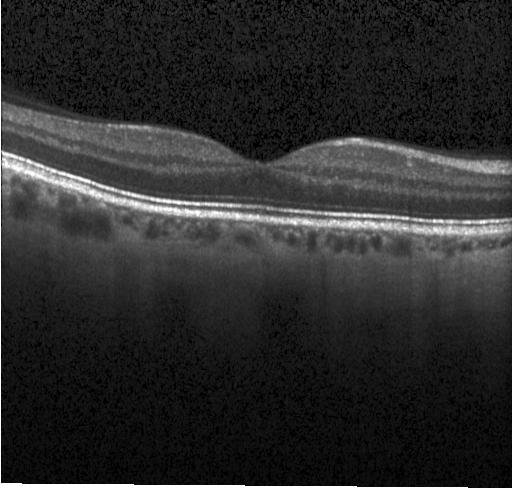 Through the macula. SD-OCT. Heidelberg Spectralis. Optical coherence tomography scan
Assessment: neither choroidal neovascularization, diabetic macular edema, nor drusen.